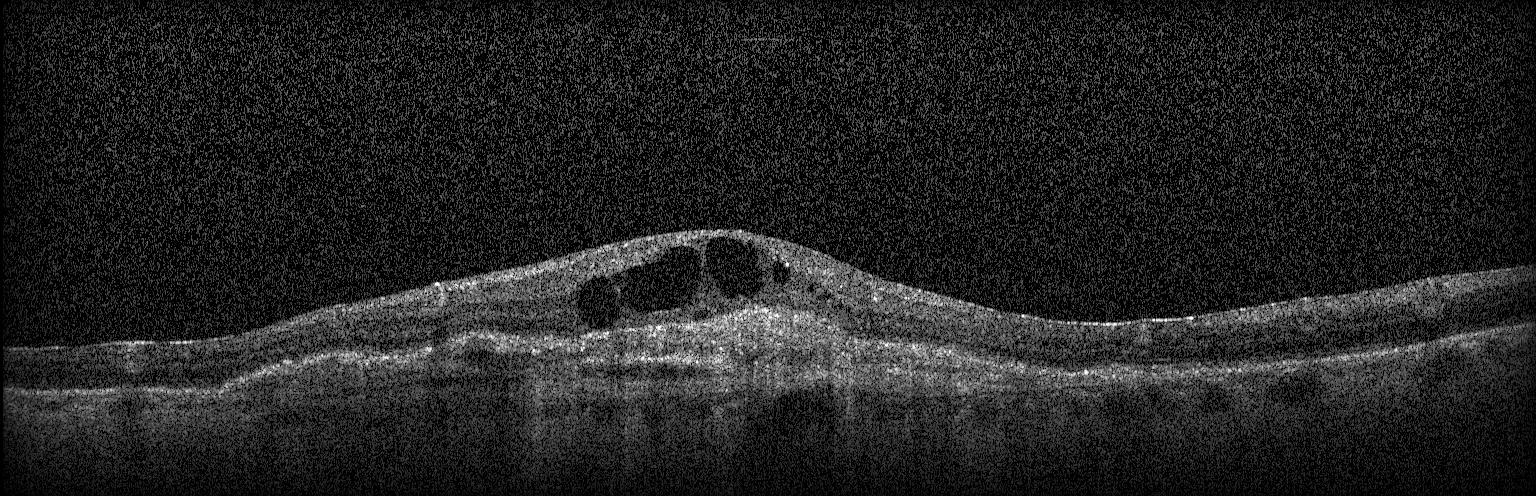
Retinal OCT cross-section.
Finding: a choroidal neovascular membrane.